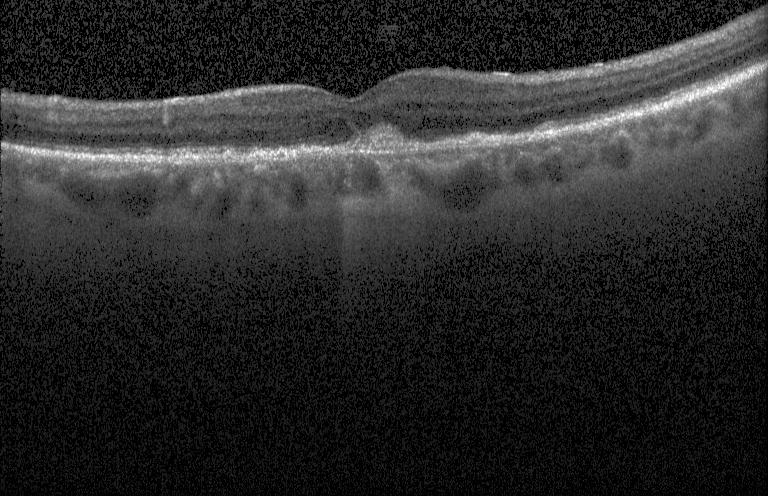 OCT line scan. Spectral-domain optical coherence tomography. Acquired on a Heidelberg Spectralis. Fovea-centered — This B-scan demonstrates CNV.